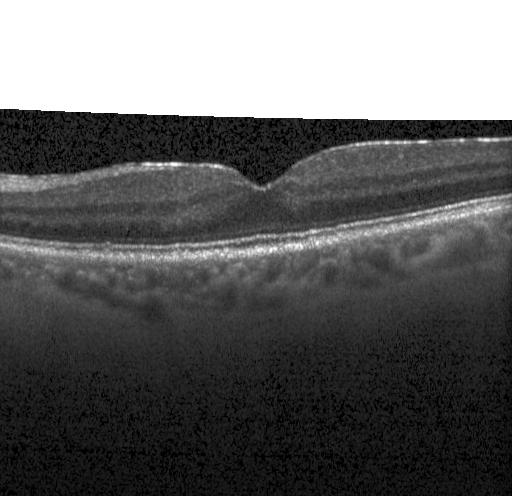

Heidelberg Spectralis; OCT line scan; spectral-domain optical coherence tomography; through the macula.
Diagnosis: no CNV, DME, or drusen.